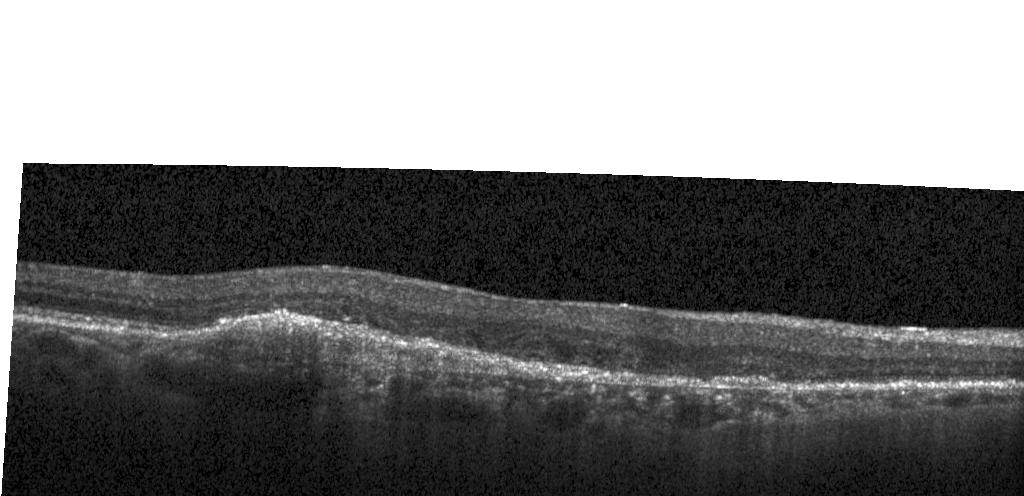

Diagnosis: choroidal neovascularization.